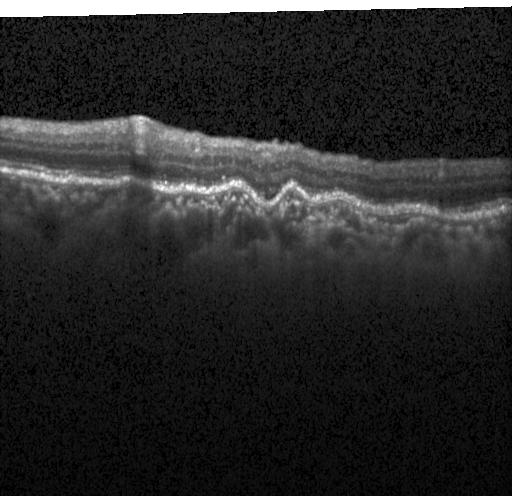

Dx: choroidal neovascularization (CNV).